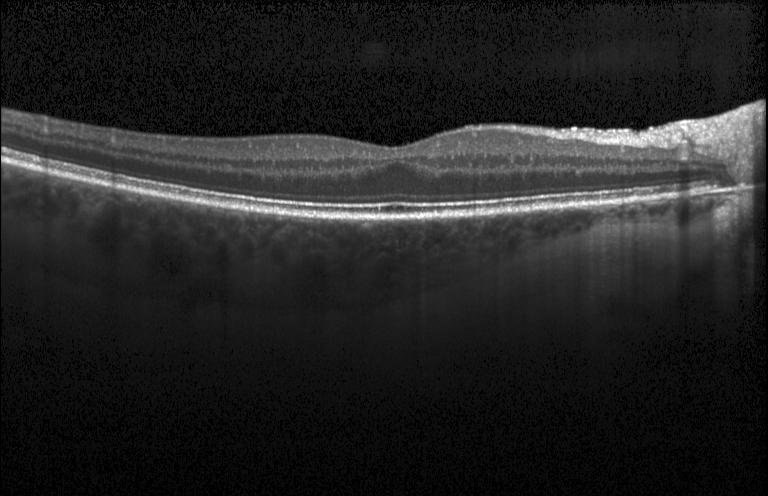
Spectral-domain OCT. Centered on the fovea. OCT line scan. Instrument: Heidelberg Spectralis
No CNV, DME, or drusen.